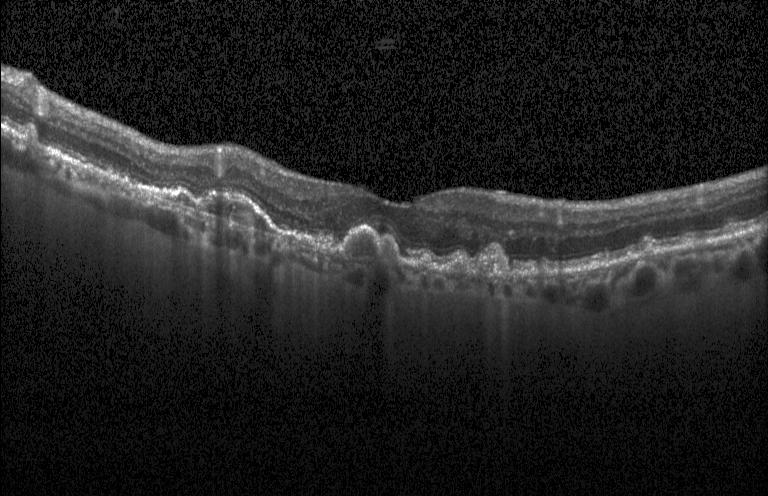 OCT finding: drusen.